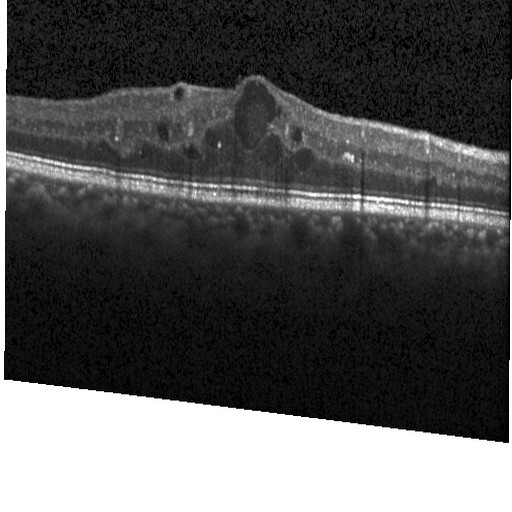

Retinal OCT cross-section · centered on the fovea — Dx: diabetic macular edema (DME).